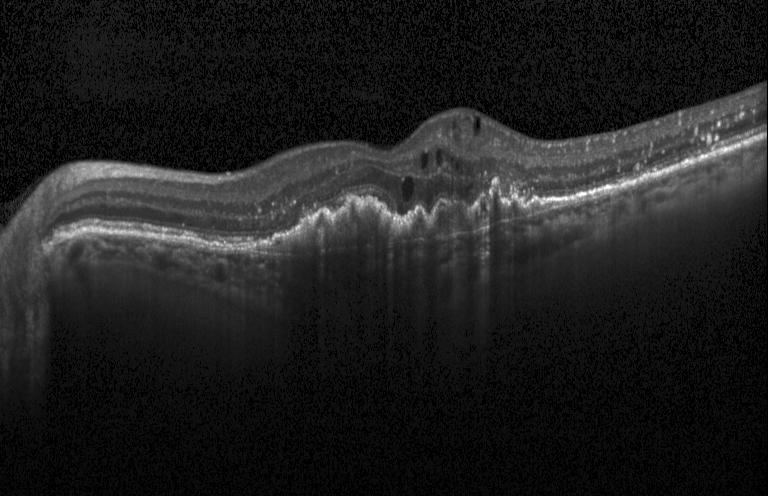 OCT line scan · centered on the fovea.
Finding: CNV.